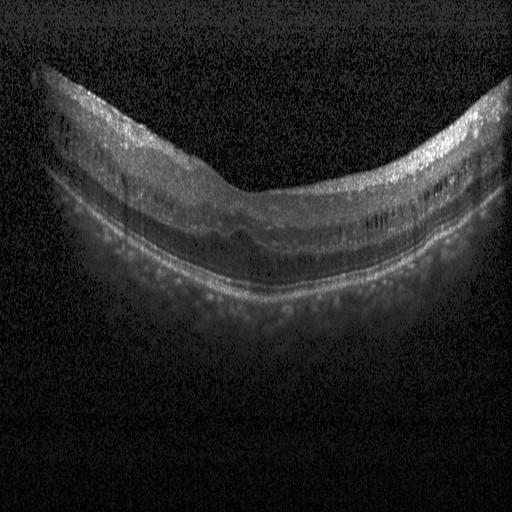 Spectral-domain OCT, through the macula, retinal OCT B-scan. This B-scan demonstrates DME.